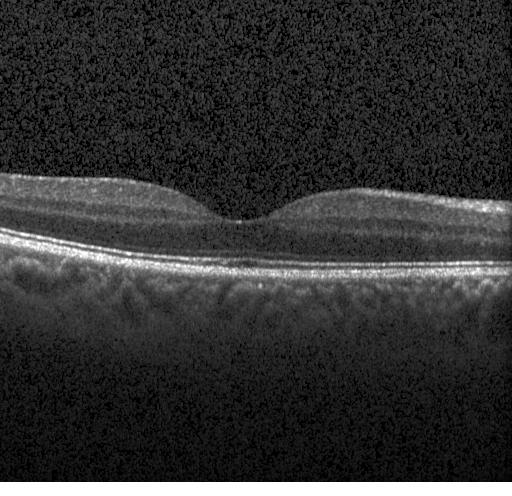

Spectral-domain OCT B-scan: no evidence of choroidal neovascularization, diabetic macular edema, or drusen.